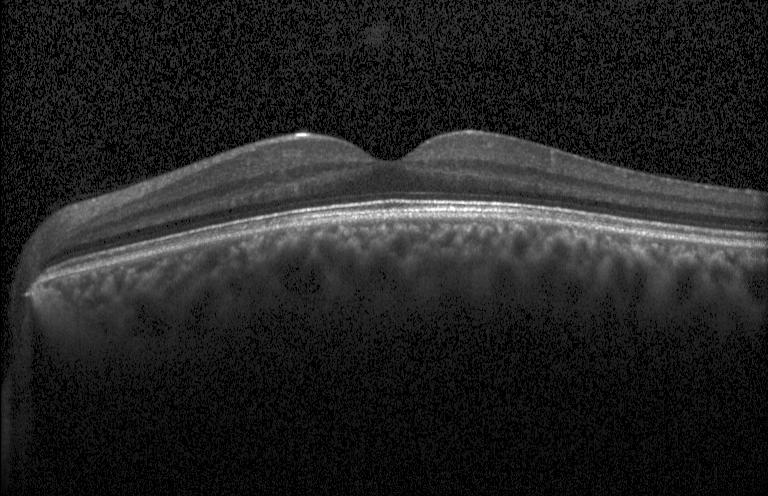

Spectral-domain OCT, optical coherence tomography scan — Macular OCT: no choroidal neovascularization, diabetic macular edema, or drusen.